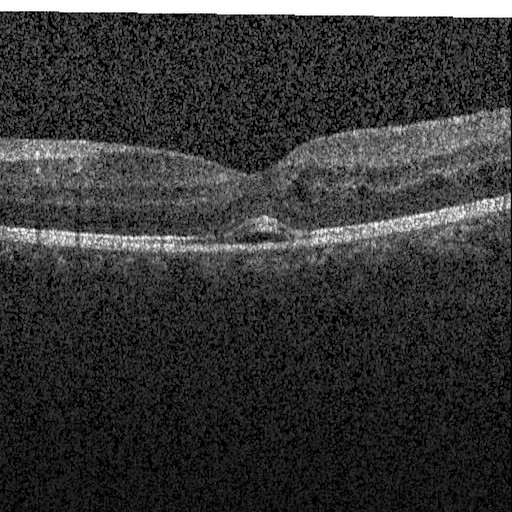
Macular OCT: DME.